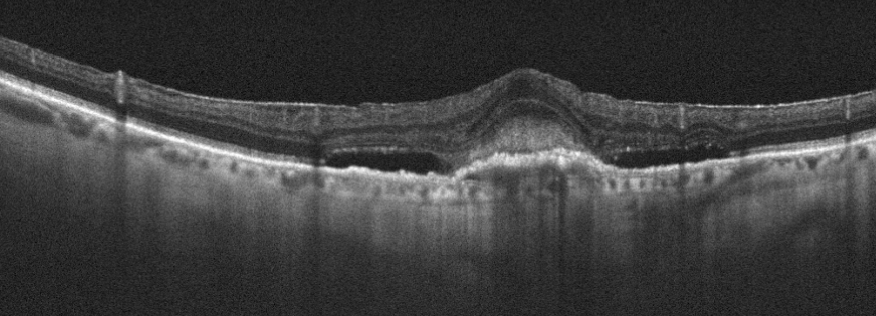
Optovue Avanti RTVue XR · OCT B-scan
Impression: age-related macular degeneration (AMD).